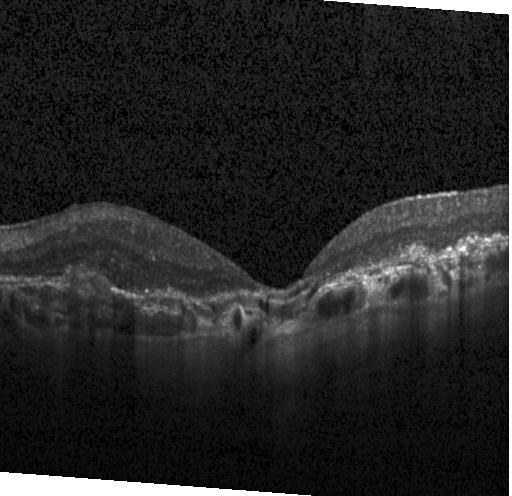 Spectral-domain optical coherence tomography. Optical coherence tomography scan. Fovea-centered. Heidelberg Spectralis — Macular OCT: a choroidal neovascular membrane.